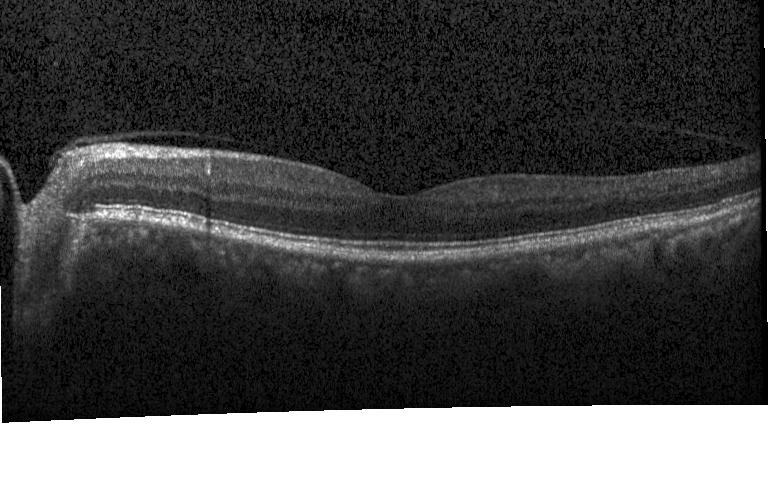
Optical coherence tomography scan; through the macula; SD-OCT; instrument: Heidelberg Spectralis — Impression: neither choroidal neovascularization, diabetic macular edema, nor drusen.